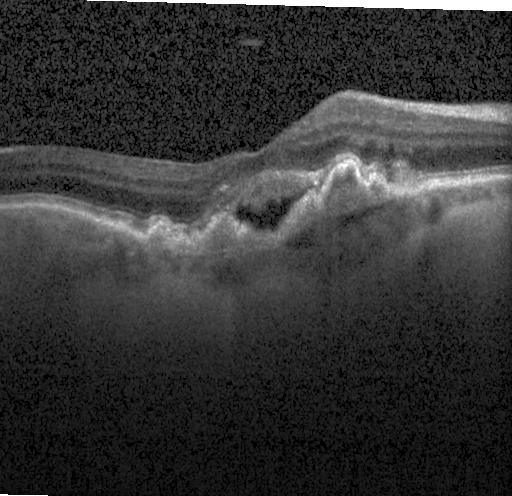

Optical coherence tomography scan.
Diagnosis: a choroidal neovascular membrane.